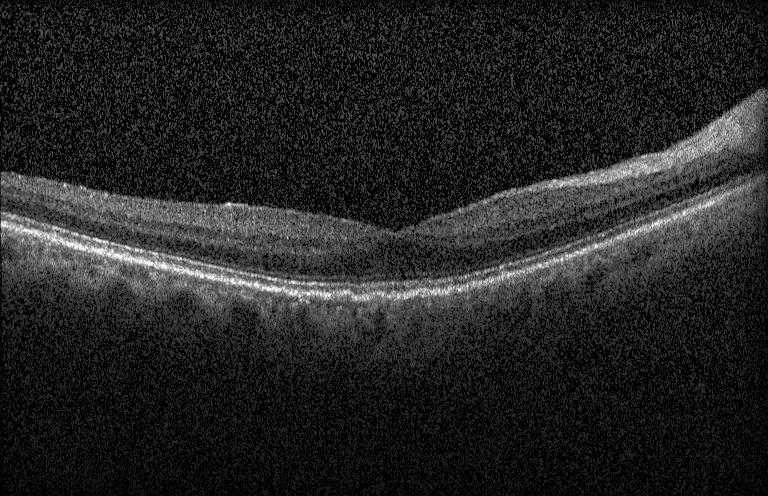 Impression: sub-RPE drusenoid deposits.